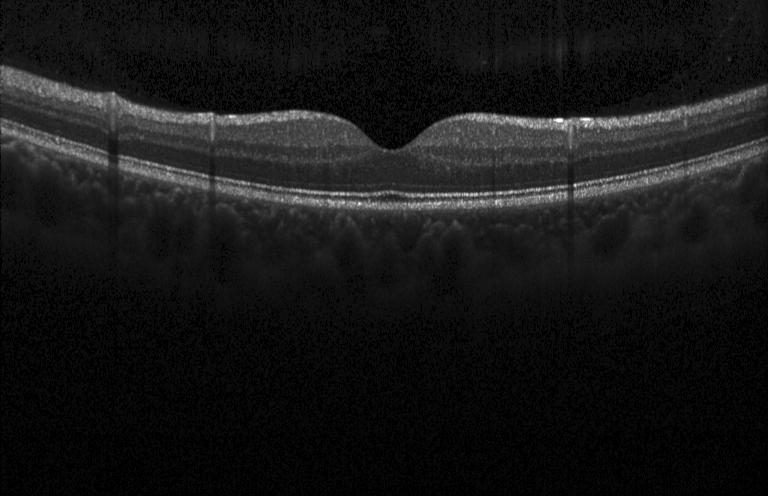

OCT finding: no choroidal neovascularization, diabetic macular edema, or drusen.